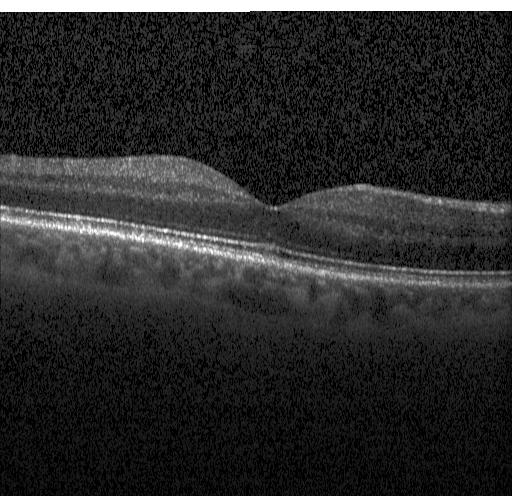

Heidelberg Spectralis · horizontal scan through the fovea · spectral-domain OCT · retinal OCT B-scan. OCT finding: no choroidal neovascularization, no diabetic macular edema, and no drusen.